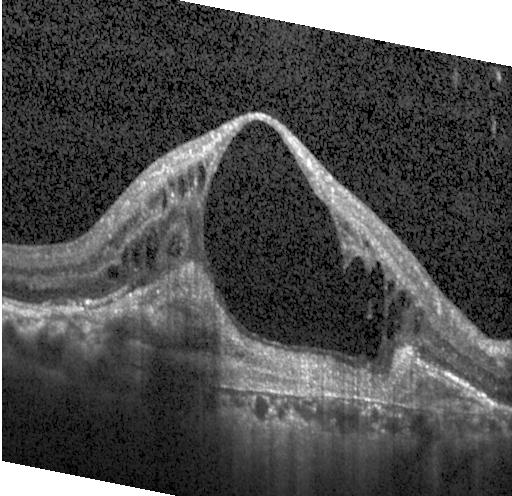 Retinal OCT cross-section. Instrument: Heidelberg Spectralis. Through the macula. This B-scan demonstrates choroidal neovascularization (CNV).